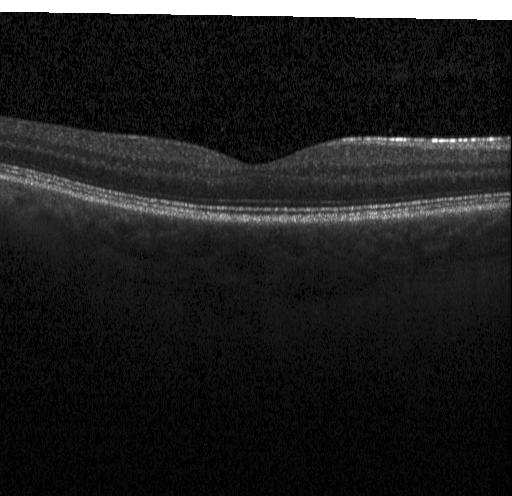 Centered on the fovea; optical coherence tomography scan; acquired on a Heidelberg Spectralis; SD-OCT.
The scan shows no evidence of choroidal neovascularization, diabetic macular edema, or drusen.